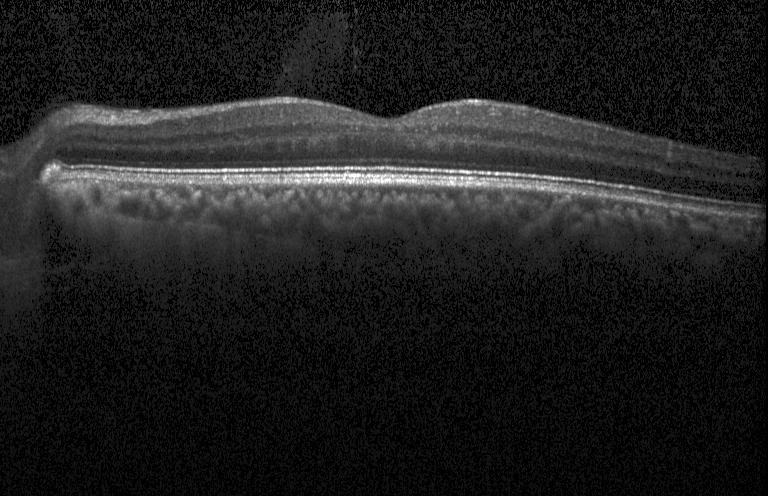
Optical coherence tomography scan
Diagnosis: no choroidal neovascularization, no diabetic macular edema, and no drusen.